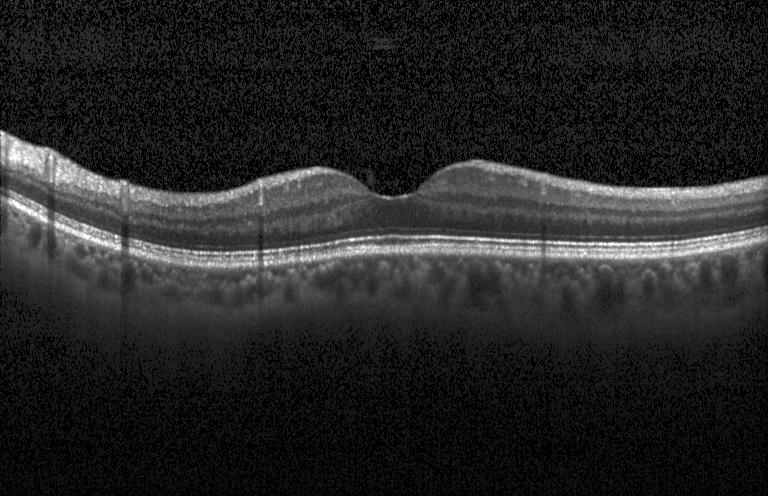

Retinal OCT cross-section. Acquired on a Heidelberg Spectralis. Spectral-domain OCT.
Diagnosis: no choroidal neovascularization, diabetic macular edema, or drusen.